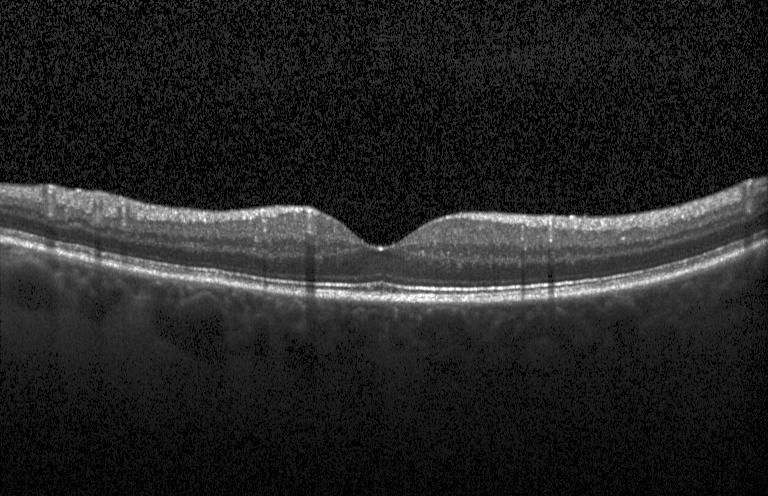
Optical coherence tomography scan. The scan shows no choroidal neovascularization, no diabetic macular edema, and no drusen.